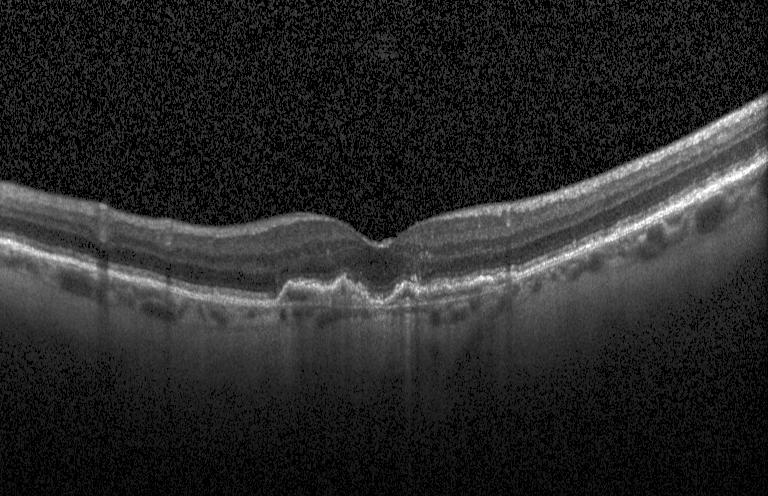 This B-scan demonstrates a choroidal neovascular membrane.